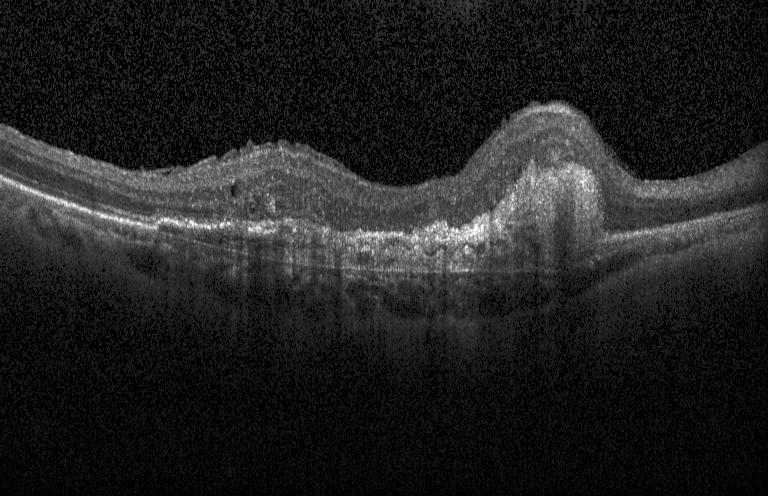
Retinal OCT cross-section showing choroidal neovascularization.